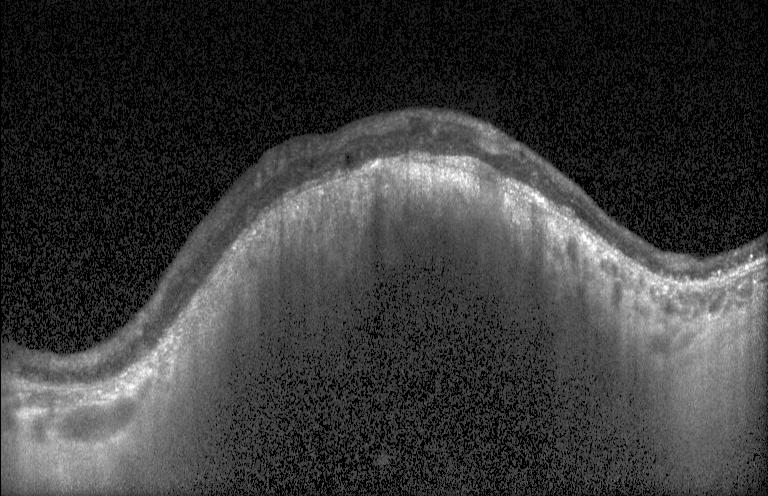
Instrument: Heidelberg Spectralis, retinal OCT cross-section, macular scan, spectral-domain OCT
Macular OCT: diabetic macular edema.